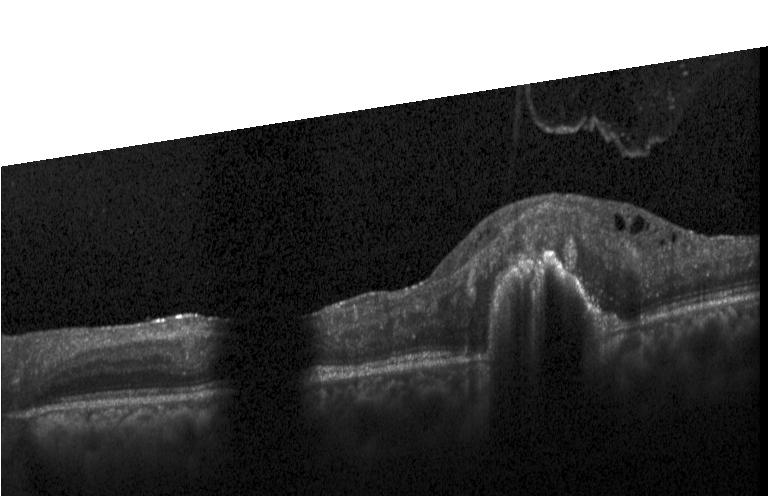

Retinal OCT cross-section showing a choroidal neovascular membrane.